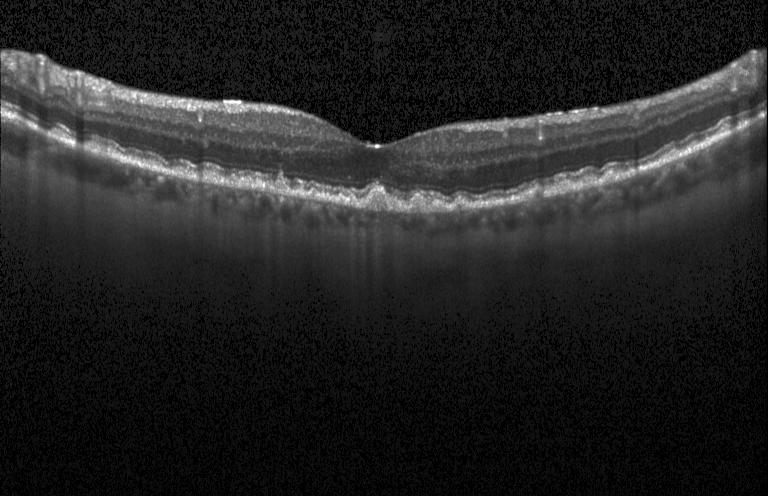
Instrument: Heidelberg Spectralis. SD-OCT. Retinal OCT B-scan — Finding: drusen.